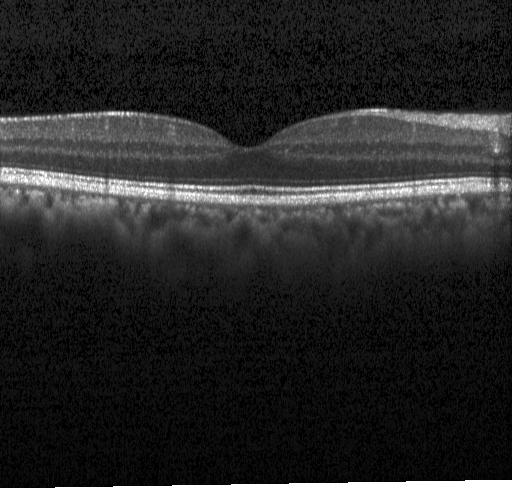 Centered on the fovea · OCT B-scan.
This B-scan demonstrates neither CNV, DME, nor drusen.